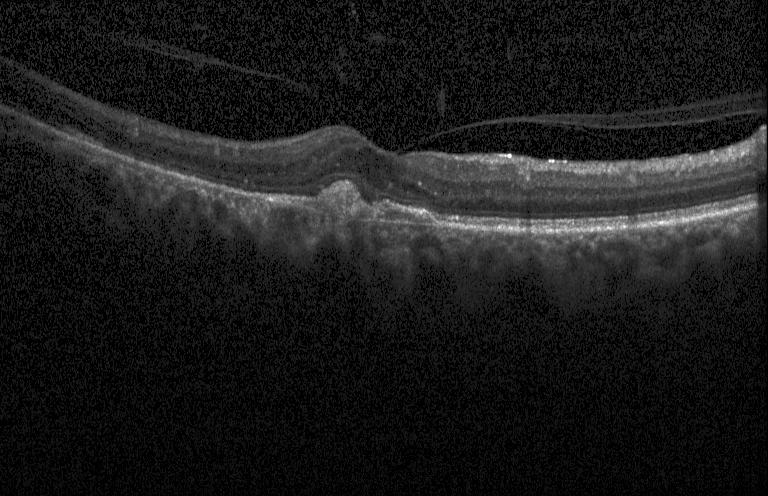 Macular OCT: CNV.